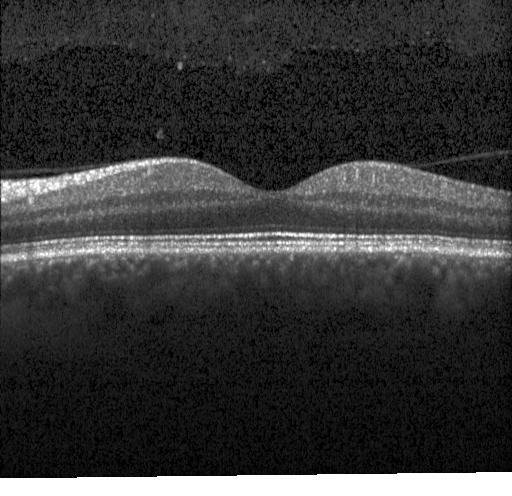 Horizontal scan through the fovea, acquired on a Heidelberg Spectralis, retinal OCT cross-section. Impression: no choroidal neovascularization, diabetic macular edema, or drusen.